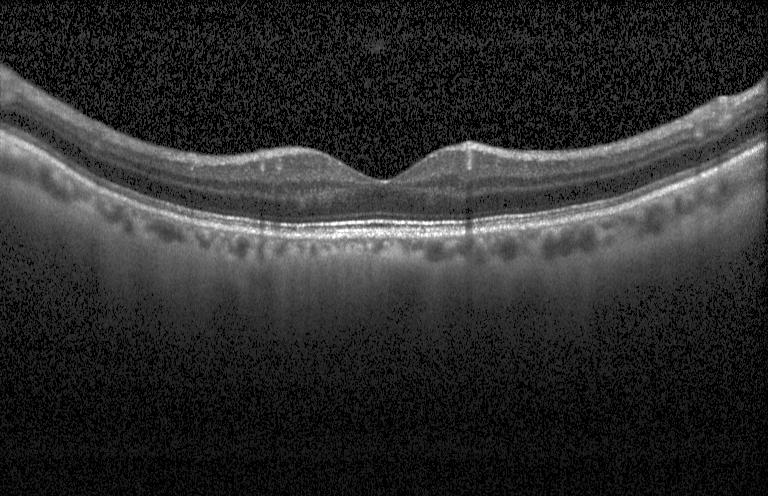
Retinal OCT cross-section. OCT finding: no CNV, DME, or drusen.